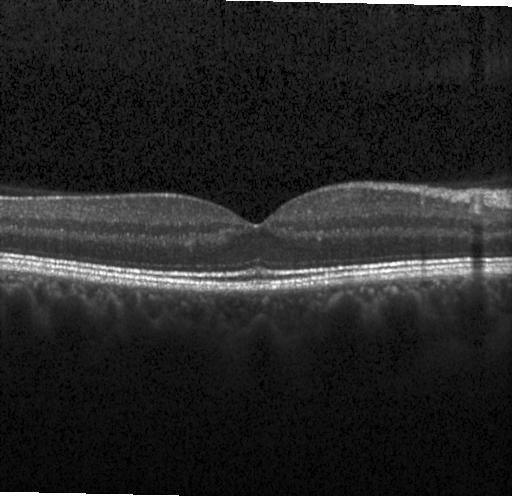 Diagnosis: no choroidal neovascularization, no diabetic macular edema, and no drusen.